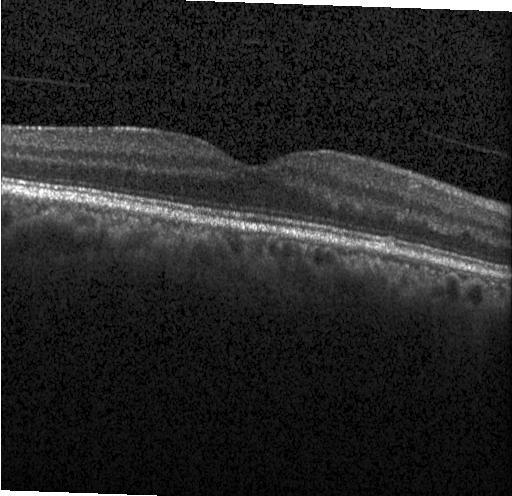

OCT B-scan, acquired on a Heidelberg Spectralis, spectral-domain optical coherence tomography. The scan shows no choroidal neovascularization, diabetic macular edema, or drusen.